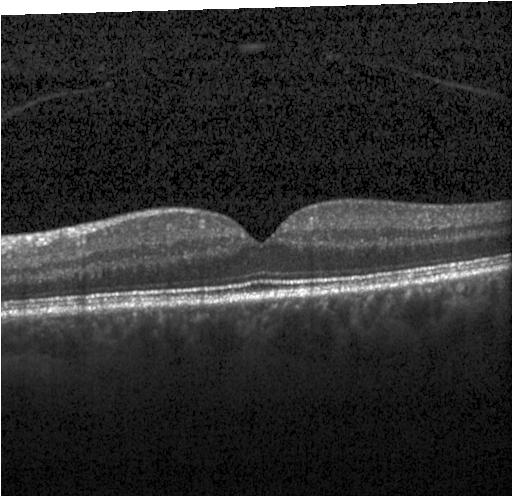

Optical coherence tomography scan — The scan shows no choroidal neovascularization, no diabetic macular edema, and no drusen.